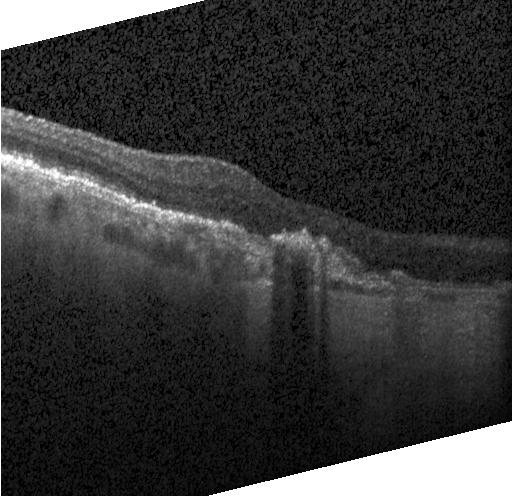 OCT B-scan. Dx: a choroidal neovascular membrane.